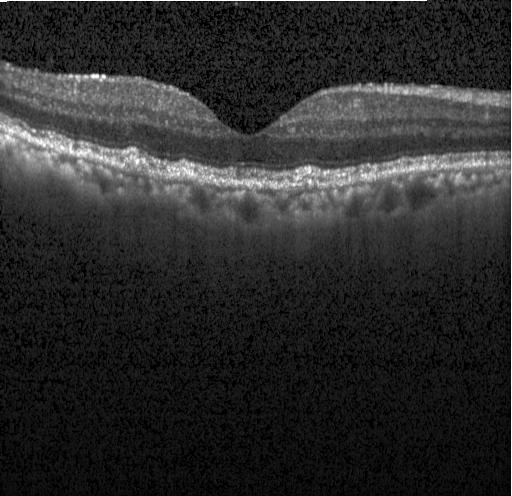

OCT line scan. Finding: sub-RPE drusenoid deposits.